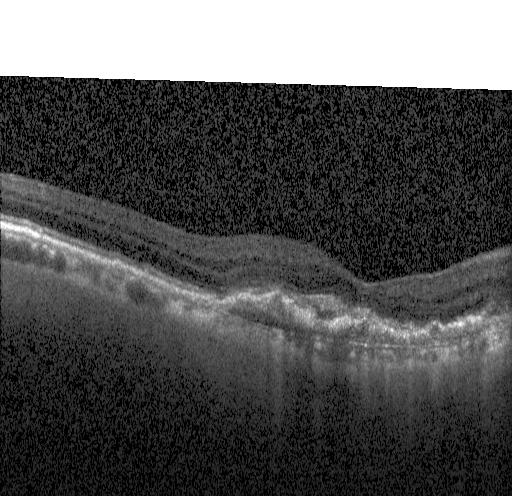

Spectral-domain OCT B-scan: a choroidal neovascular membrane.